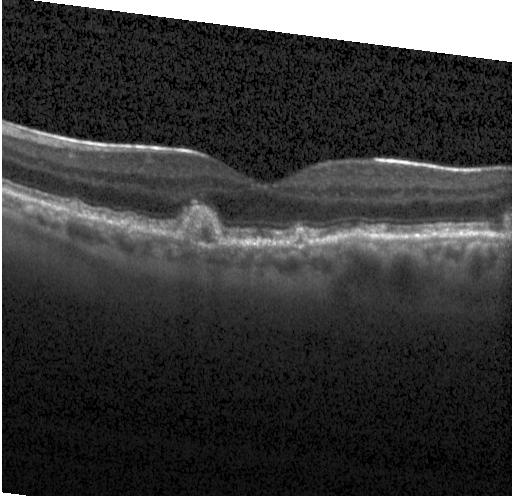
The scan shows a choroidal neovascular membrane.